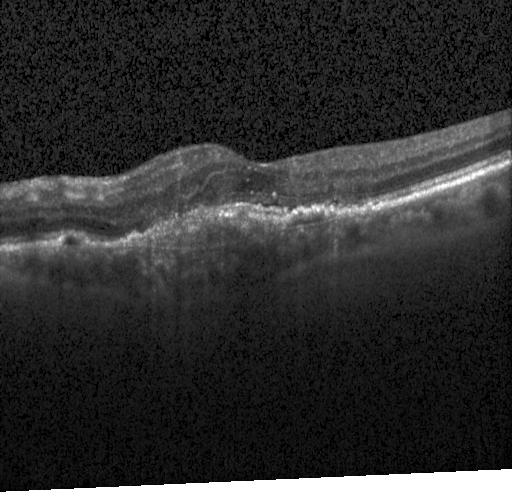 Fovea-centered; OCT B-scan
Diagnosis: a choroidal neovascular membrane.